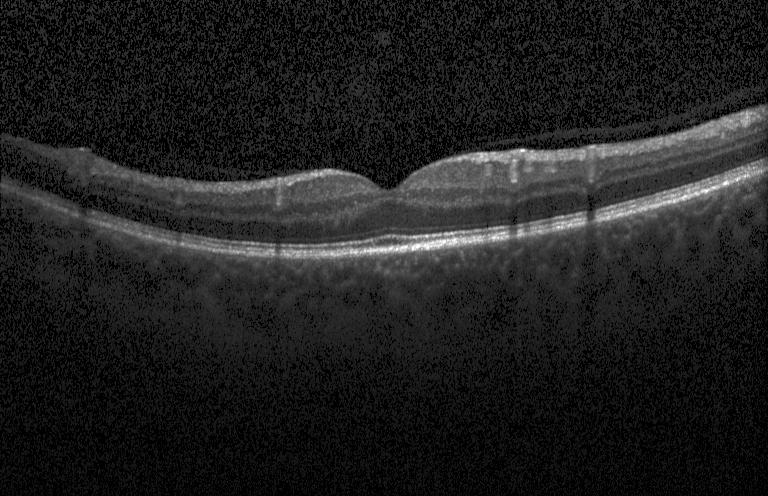

Instrument: Heidelberg Spectralis, OCT B-scan. Impression: no evidence of CNV, DME, or drusen.